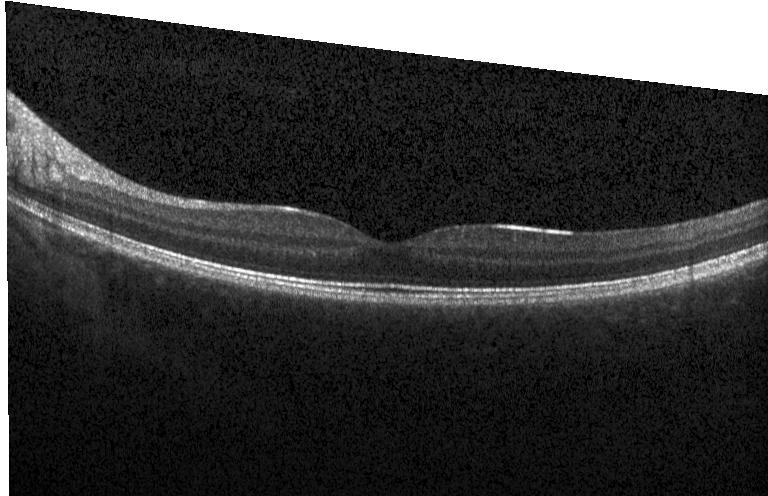 Acquired on a Heidelberg Spectralis; OCT line scan; spectral-domain OCT.
Assessment: no CNV, DME, or drusen.